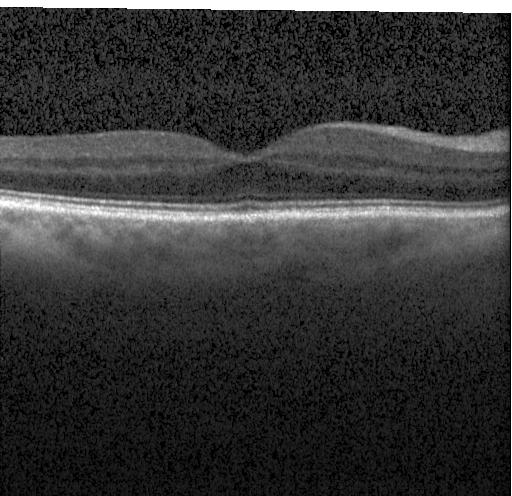

OCT finding: no choroidal neovascularization, no diabetic macular edema, and no drusen.